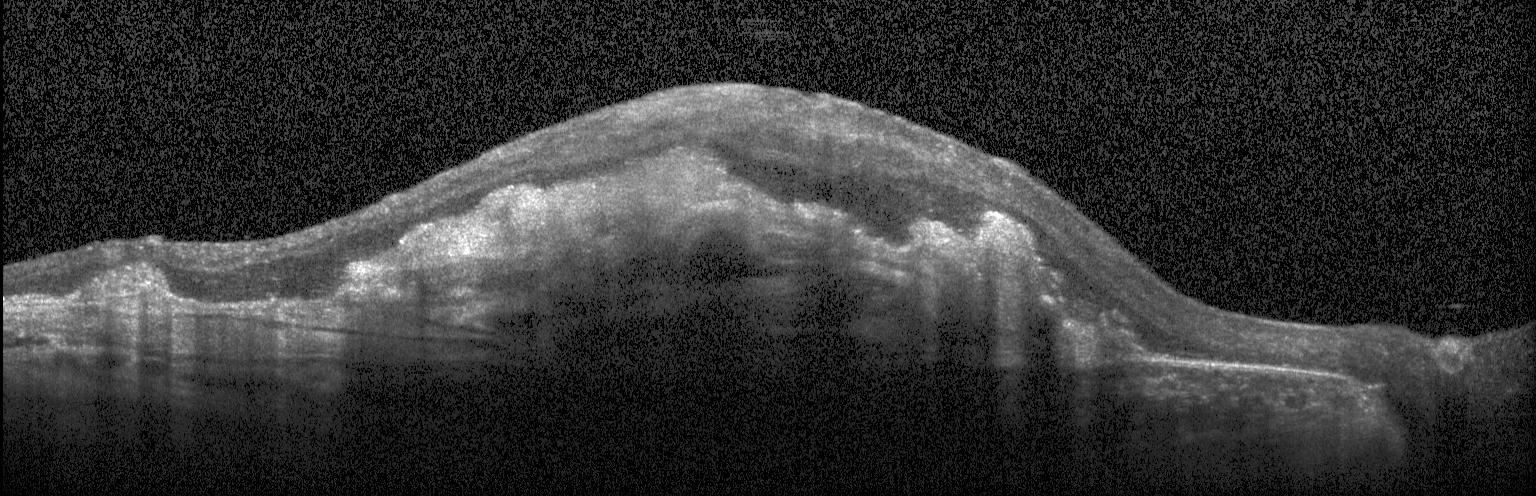

Retinal OCT cross-section, horizontal scan through the fovea.
Diagnosis: choroidal neovascularization.